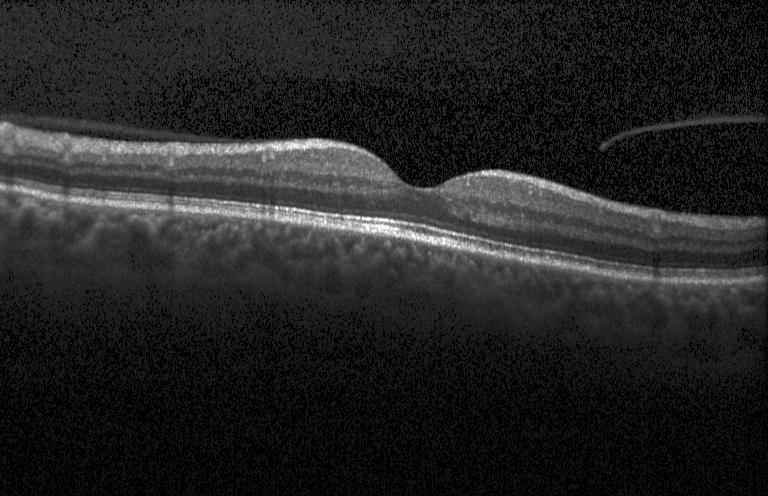 OCT scan showing no evidence of CNV, DME, or drusen.